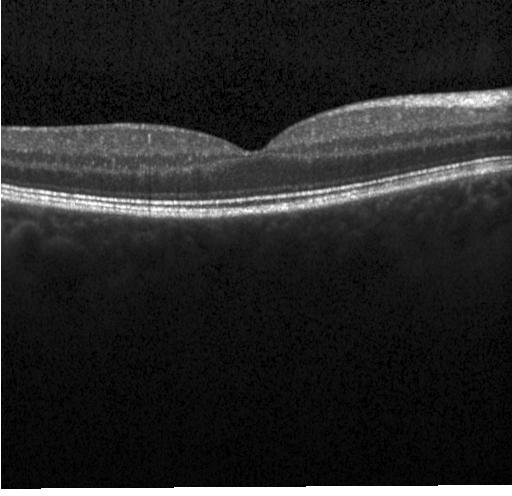 Impression: neither choroidal neovascularization, diabetic macular edema, nor drusen.